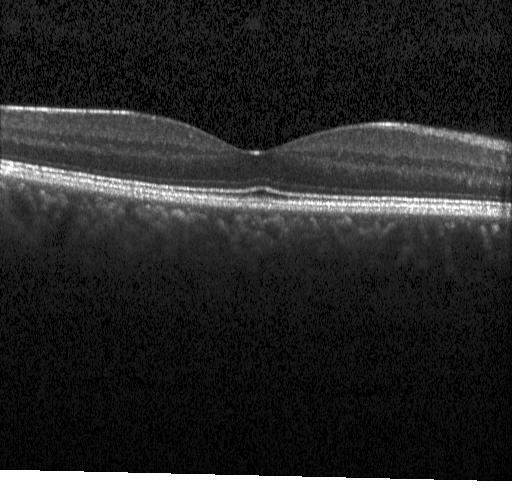 OCT finding: no evidence of CNV, DME, or drusen.